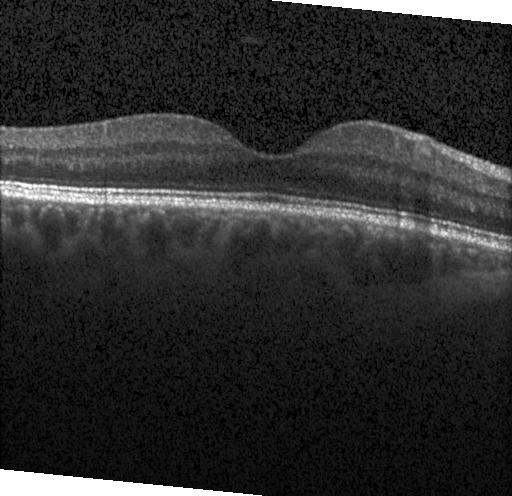

Horizontal scan through the fovea; spectral-domain optical coherence tomography; retinal OCT B-scan
Impression: no choroidal neovascularization, diabetic macular edema, or drusen.